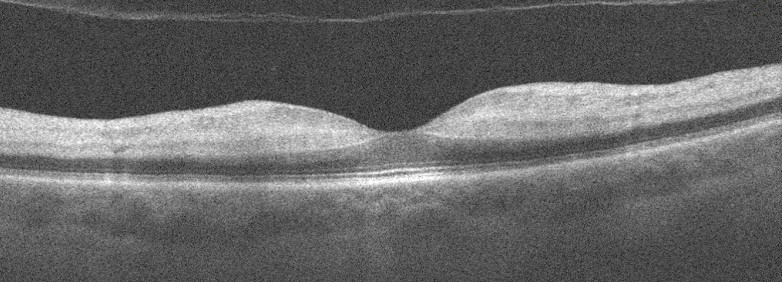
Macular OCT demonstrating RAO.